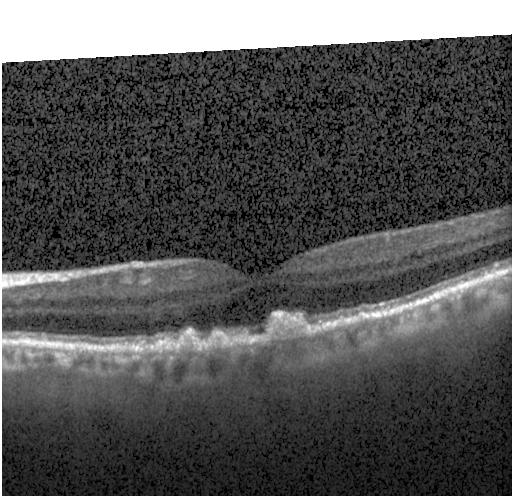 OCT B-scan showing multiple drusen.